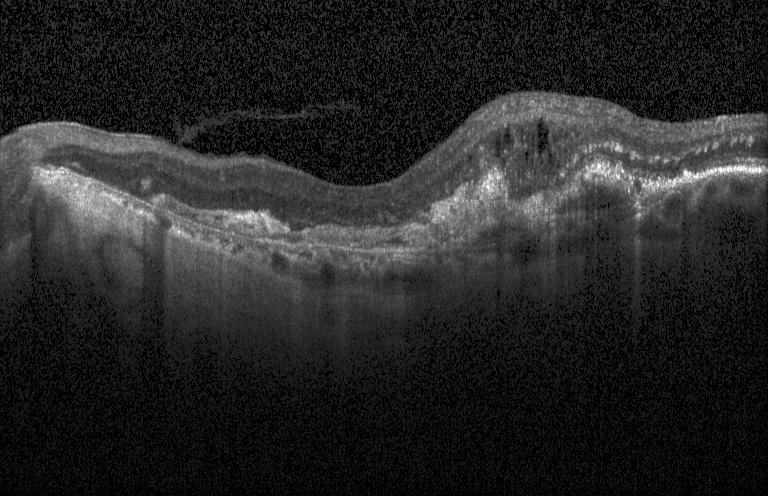 The scan shows a choroidal neovascular membrane.